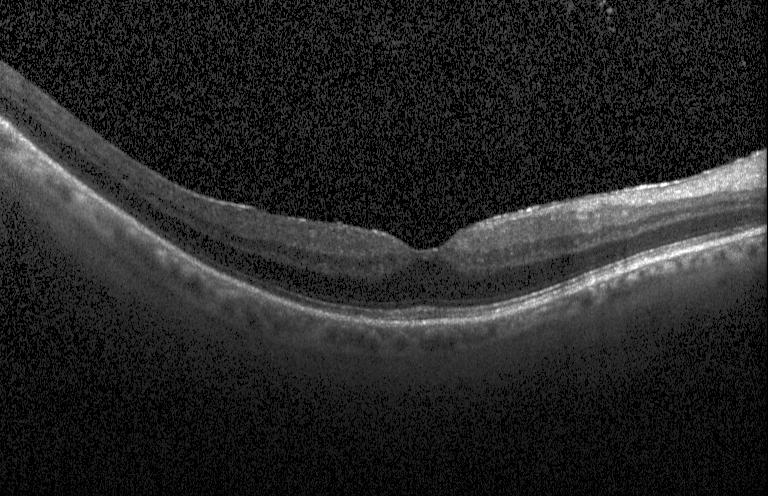 Dx: no choroidal neovascularization, diabetic macular edema, or drusen.